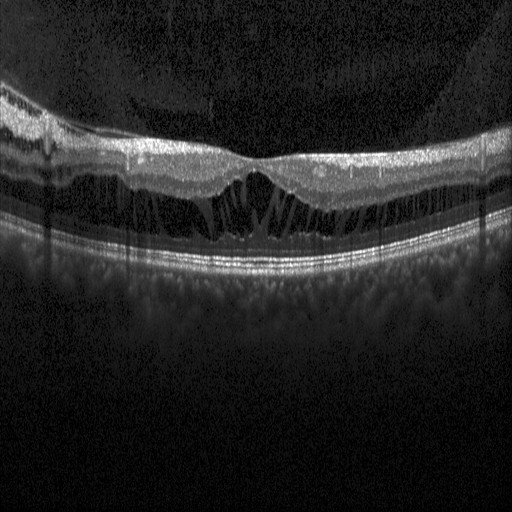
Spectral-domain OCT; retinal OCT cross-section; Heidelberg Spectralis; centered on the fovea.
This B-scan demonstrates diabetic macular edema.